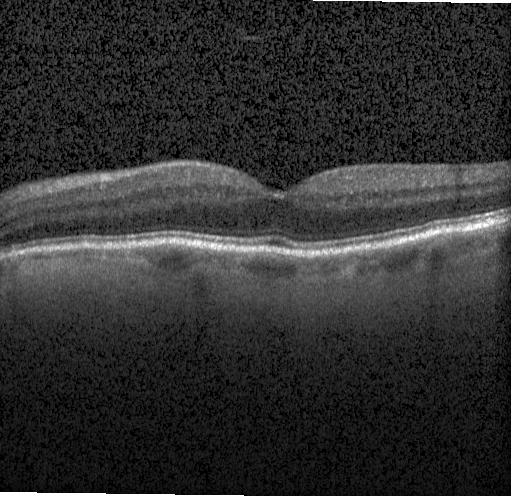

Through the macula. OCT B-scan
Finding: no choroidal neovascularization, no diabetic macular edema, and no drusen.